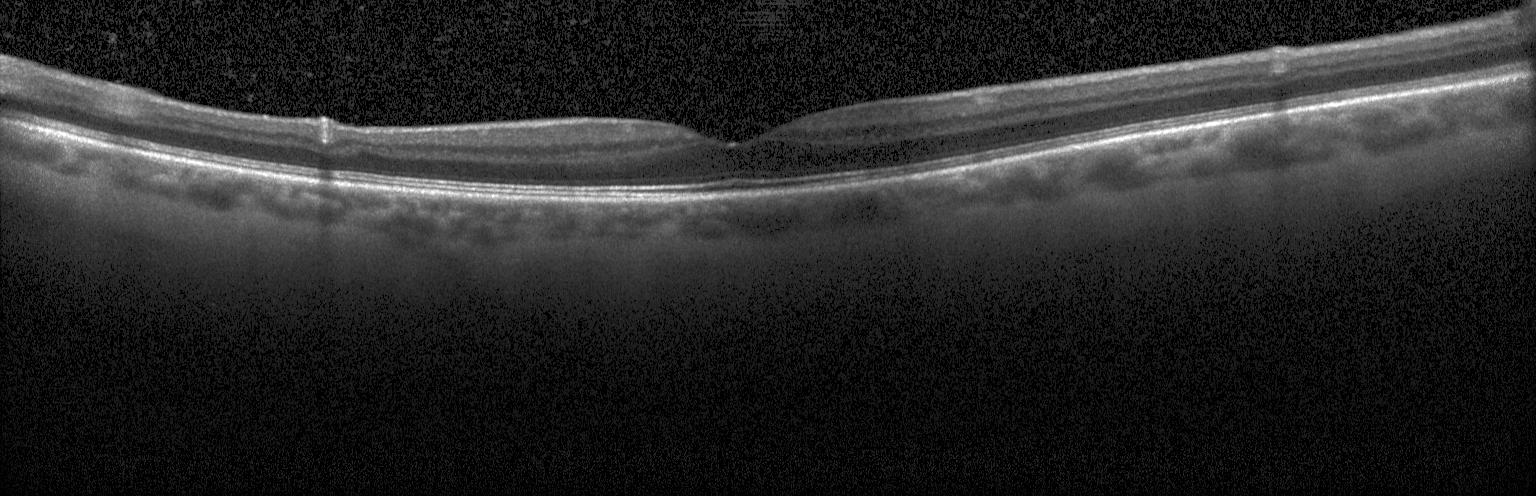

Spectral-domain optical coherence tomography; retinal OCT cross-section; Heidelberg Spectralis; centered on the fovea
Macular OCT: no choroidal neovascularization, diabetic macular edema, or drusen.